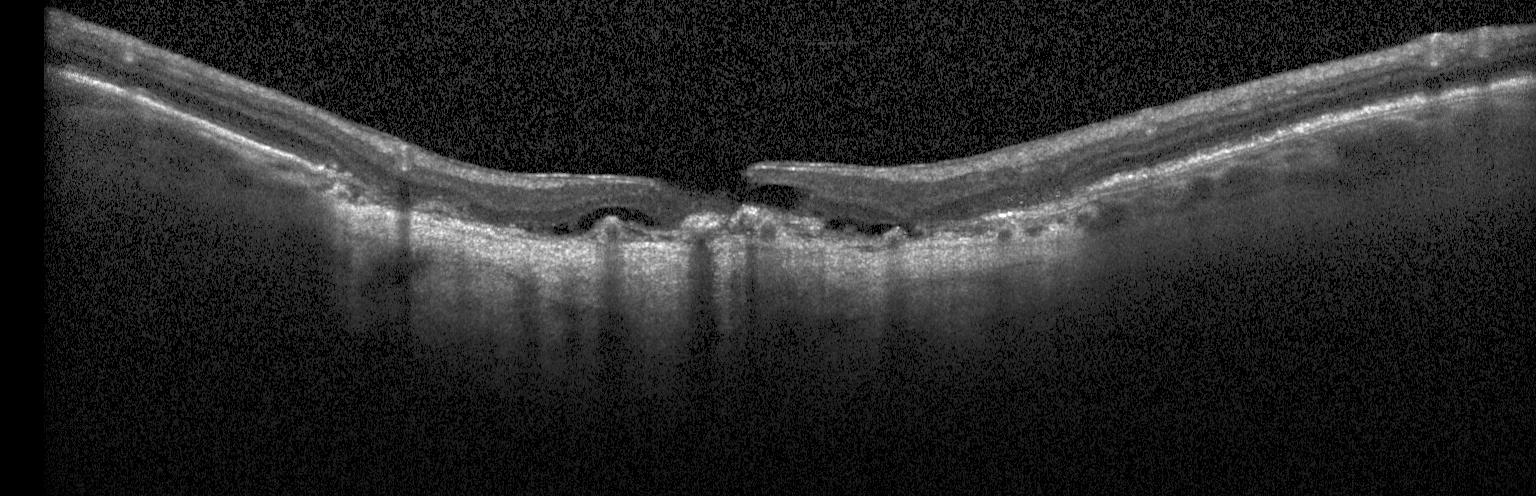

Assessment: a choroidal neovascular membrane.